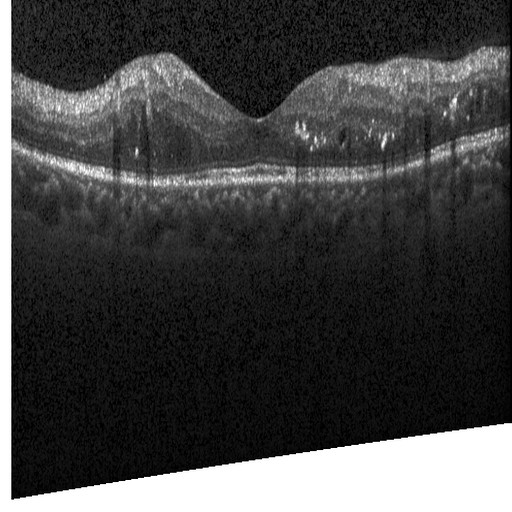 Spectral-domain optical coherence tomography, retinal OCT cross-section
Diagnosis: DME.